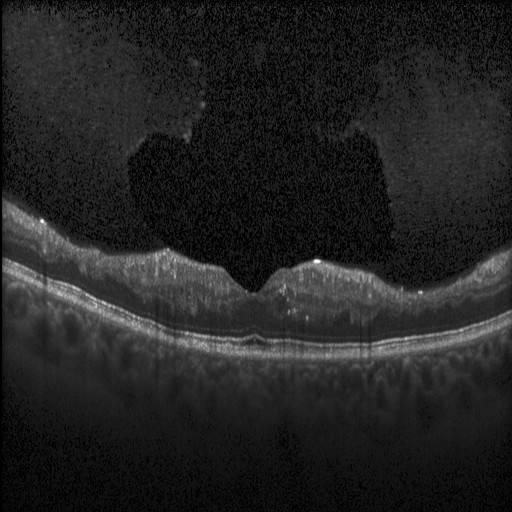
Retinal OCT cross-section · instrument: Heidelberg Spectralis · centered on the fovea
Dx: DME.